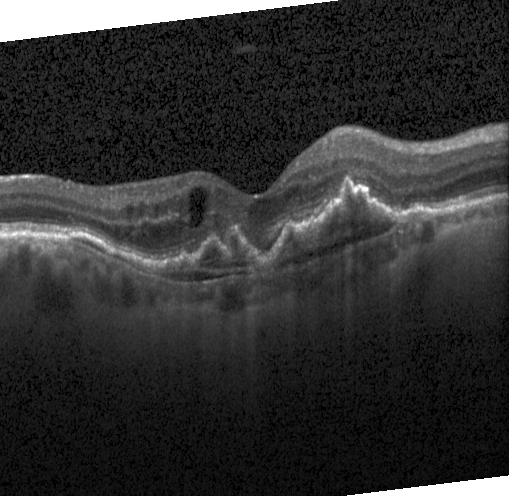
Instrument: Heidelberg Spectralis, retinal OCT cross-section, centered on the fovea
Finding: a choroidal neovascular membrane.